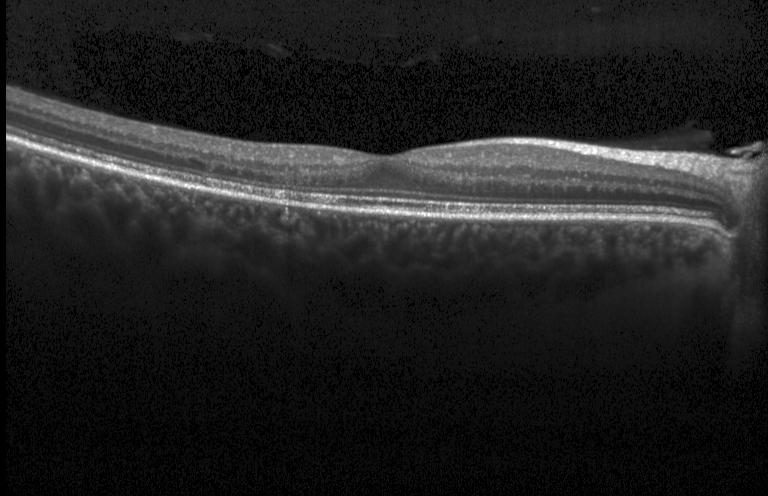 Heidelberg Spectralis OCT system; optical coherence tomography scan; horizontal scan through the fovea
Diagnosis: neither CNV, DME, nor drusen.